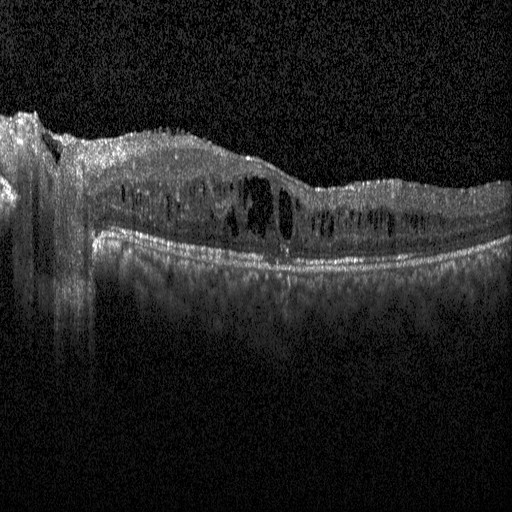

Diagnosis: DME.